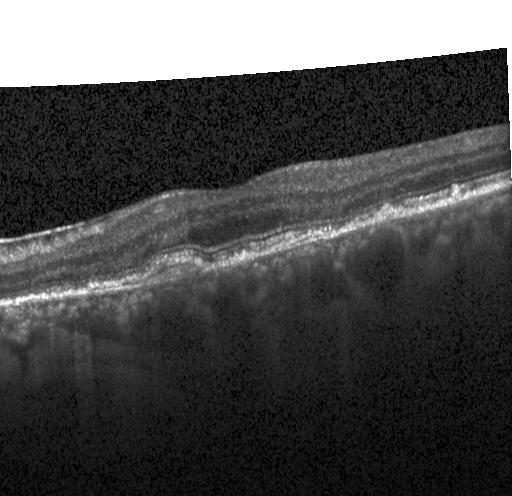
Spectral-domain OCT · retinal OCT cross-section · macular scan · instrument: Heidelberg Spectralis. Dx: choroidal neovascularization.